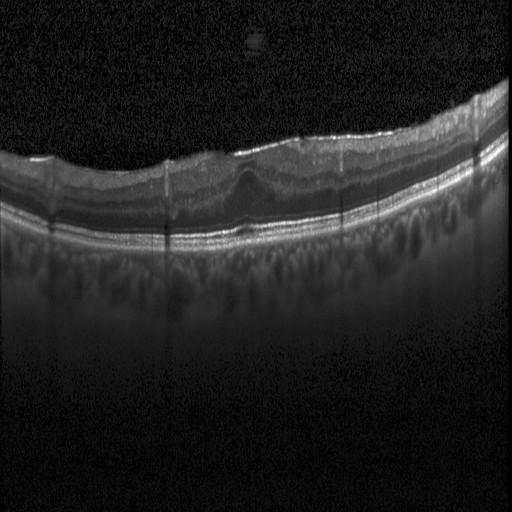

Diagnosis: DME.